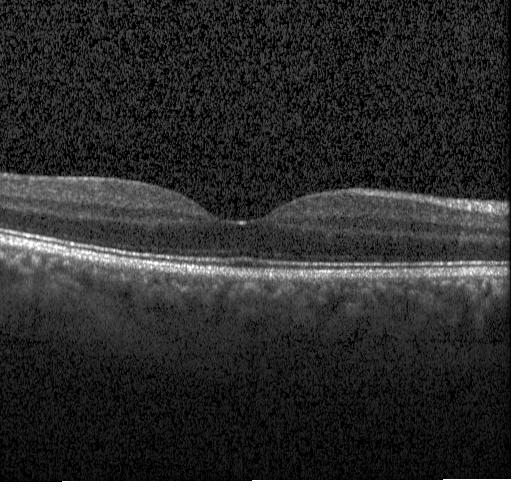
Macular OCT: no choroidal neovascularization, diabetic macular edema, or drusen.